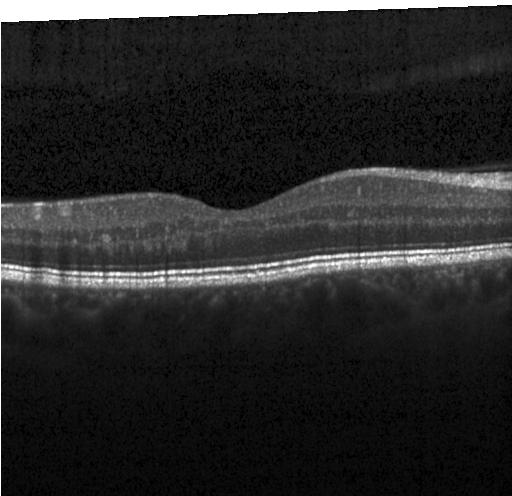
Retinal OCT cross-section, centered on the fovea, SD-OCT.
Macular OCT: neither choroidal neovascularization, diabetic macular edema, nor drusen.